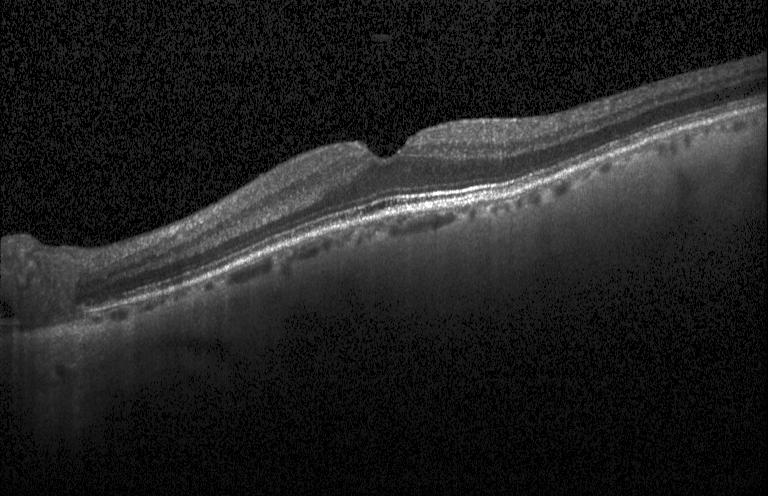

Retinal OCT B-scan; fovea-centered; spectral-domain optical coherence tomography
Dx: no evidence of choroidal neovascularization, diabetic macular edema, or drusen.